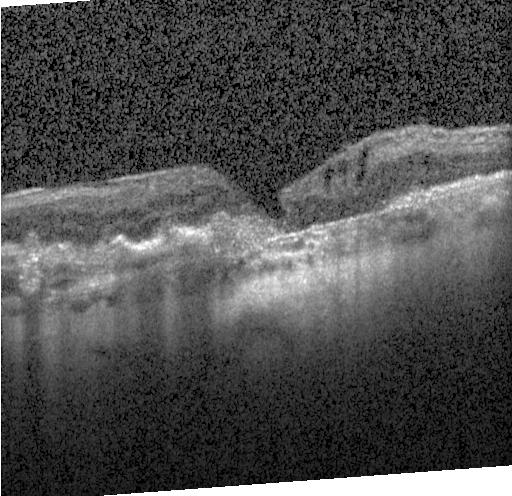
This B-scan demonstrates CNV.